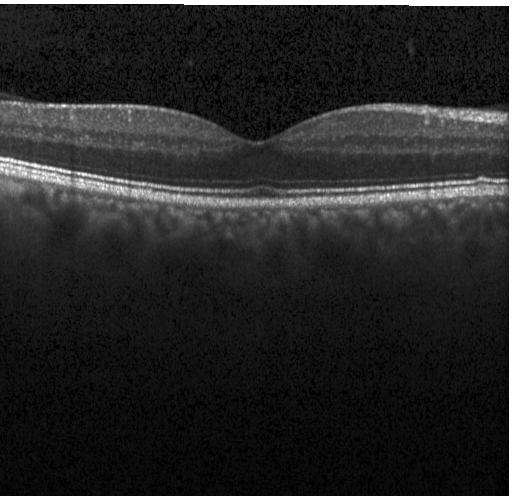 Macular scan; OCT line scan; SD-OCT. Diagnosis: neither choroidal neovascularization, diabetic macular edema, nor drusen.